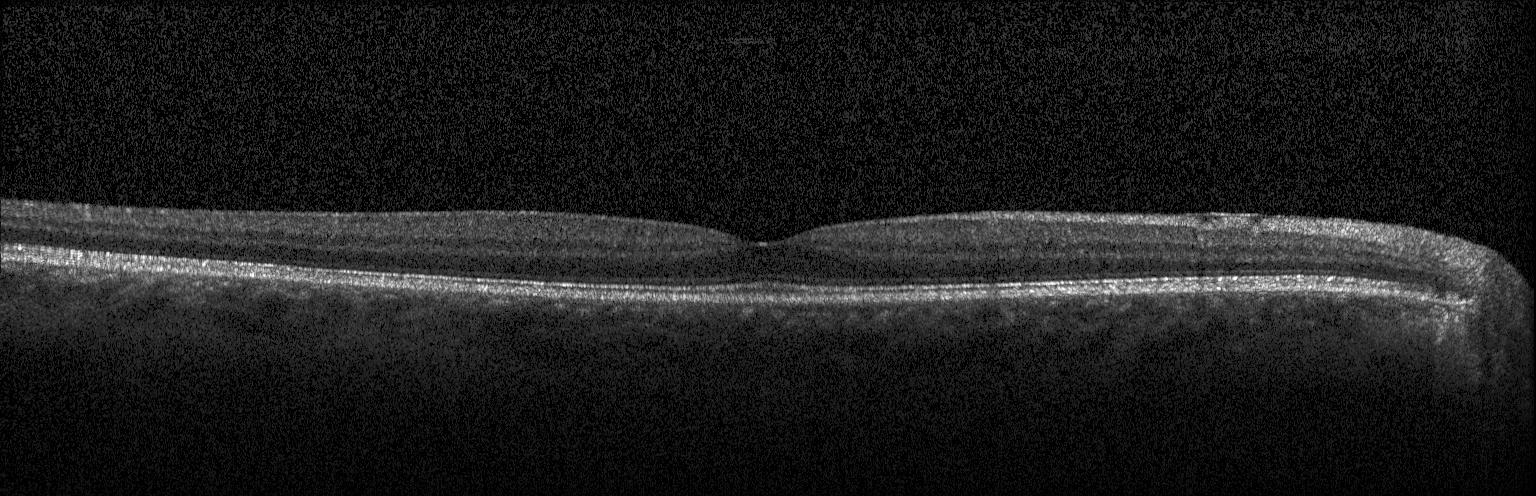
Macular scan. Optical coherence tomography B-scan.
Macular OCT: no evidence of CNV, DME, or drusen.